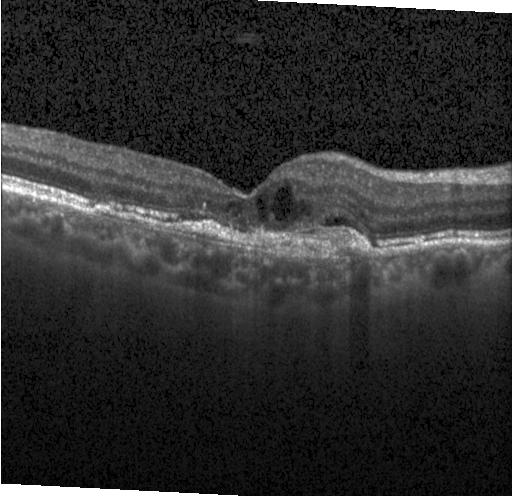 SD-OCT, centered on the fovea, optical coherence tomography B-scan — The scan shows choroidal neovascularization.